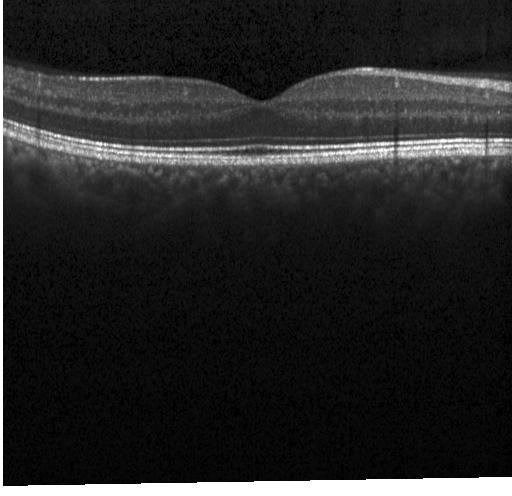
OCT line scan. Spectral-domain optical coherence tomography. Macular OCT: no evidence of choroidal neovascularization, diabetic macular edema, or drusen.